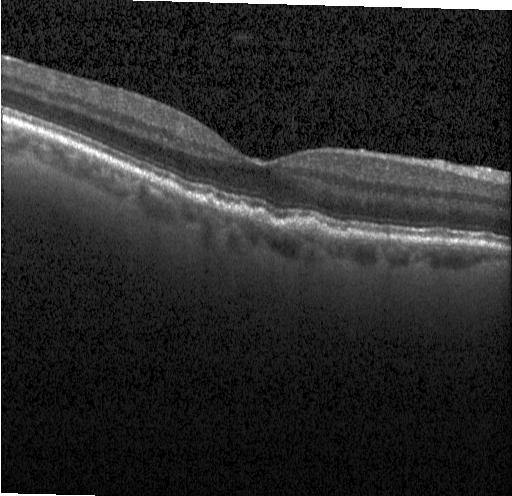 Spectral-domain OCT B-scan: sub-RPE drusenoid deposits.